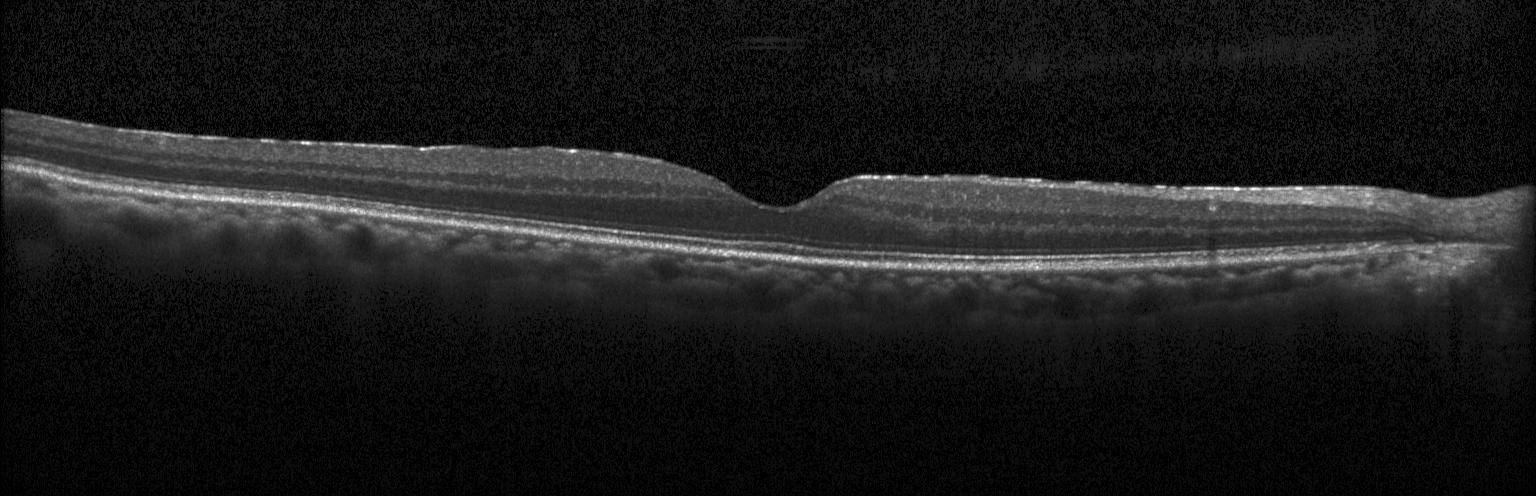 Retinal OCT cross-section showing no choroidal neovascularization, no diabetic macular edema, and no drusen.